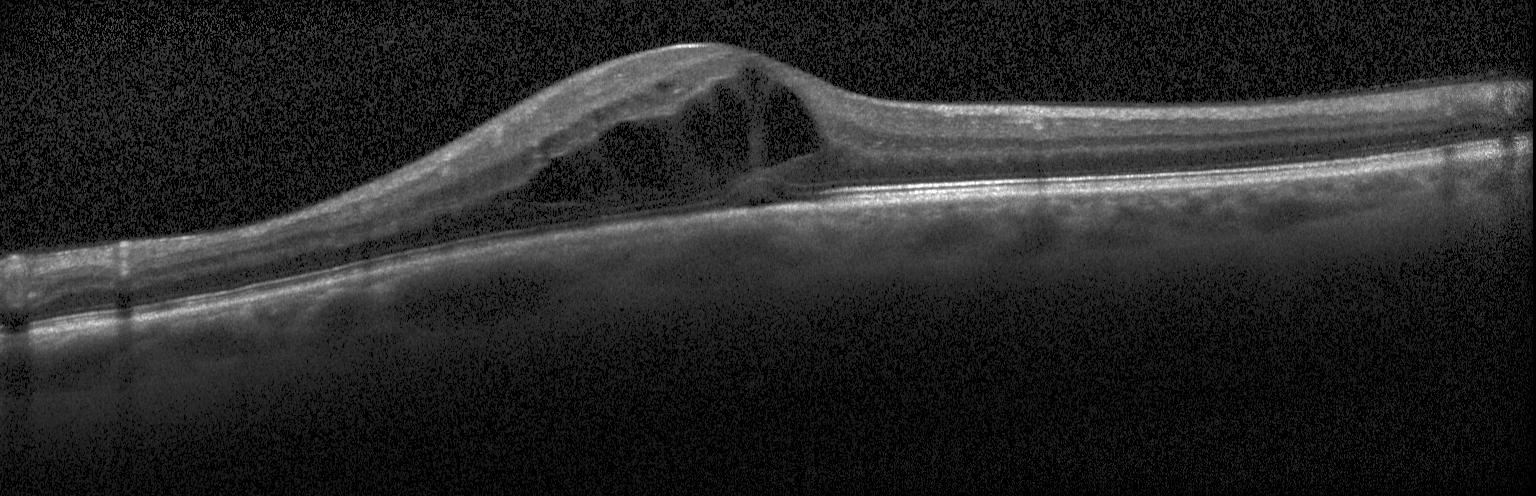

Diabetic macular edema (DME).